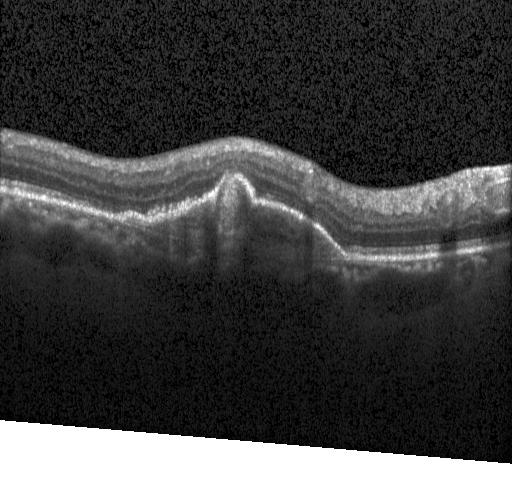

Spectral-domain OCT; acquired on a Heidelberg Spectralis; OCT line scan
Finding: choroidal neovascularization.